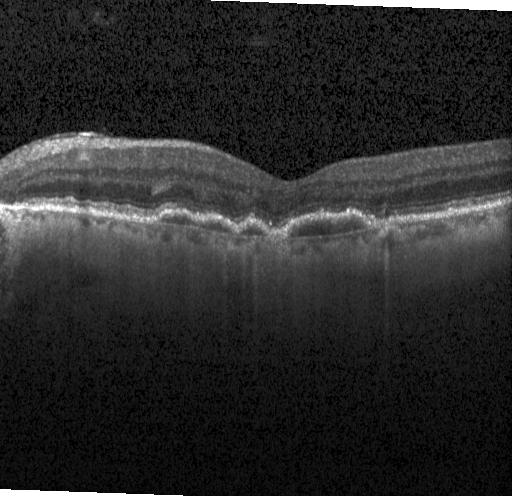 Optical coherence tomography scan · spectral-domain optical coherence tomography
The scan shows choroidal neovascularization (CNV).